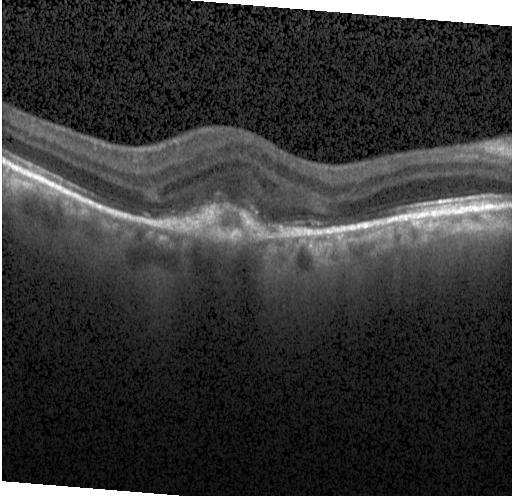 Diagnosis: CNV.